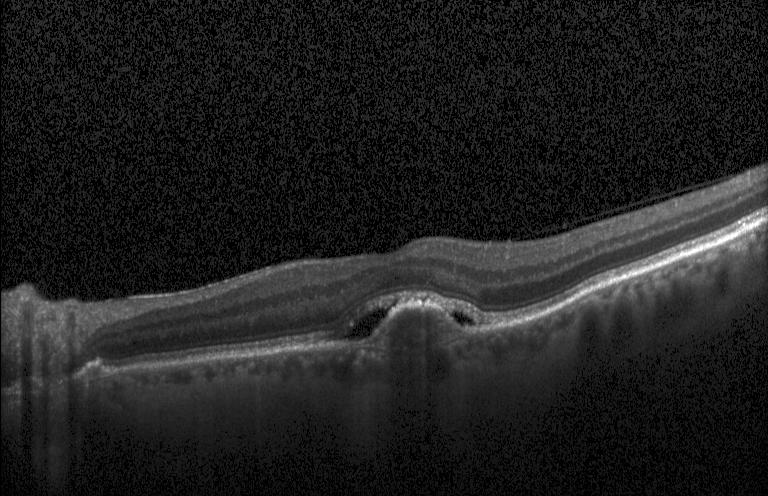 This B-scan demonstrates a choroidal neovascular membrane.